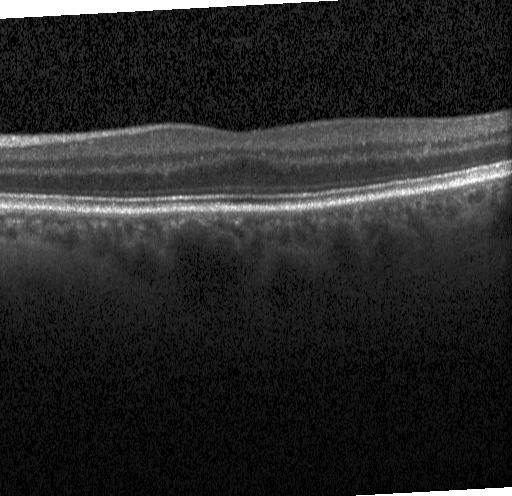
Impression: neither choroidal neovascularization, diabetic macular edema, nor drusen.